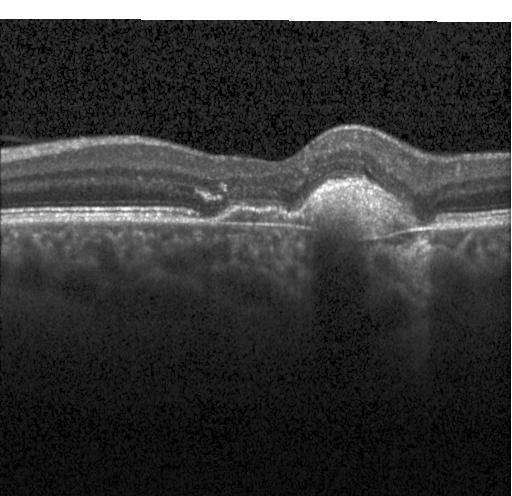
OCT finding: CNV.